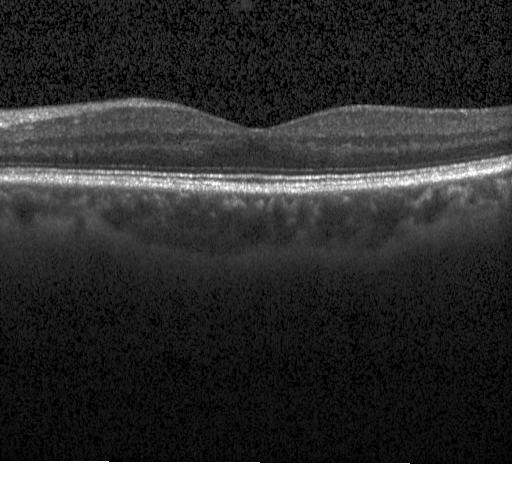
Instrument: Heidelberg Spectralis; optical coherence tomography B-scan — Diagnosis: no choroidal neovascularization, diabetic macular edema, or drusen.